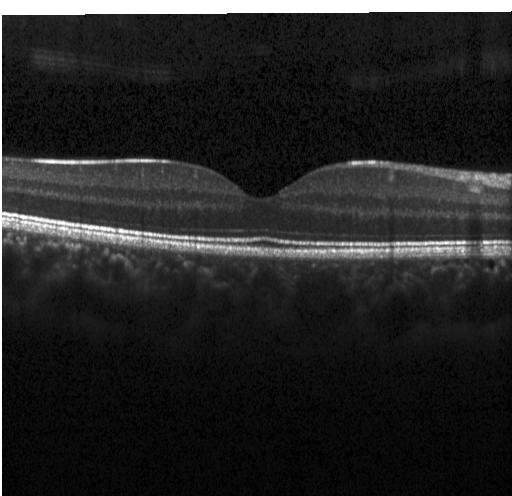
OCT B-scan. Horizontal scan through the fovea.
OCT finding: no choroidal neovascularization, diabetic macular edema, or drusen.